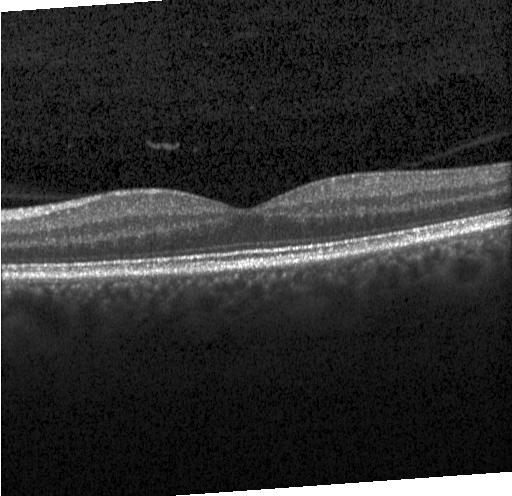
OCT B-scan showing no choroidal neovascularization, diabetic macular edema, or drusen.